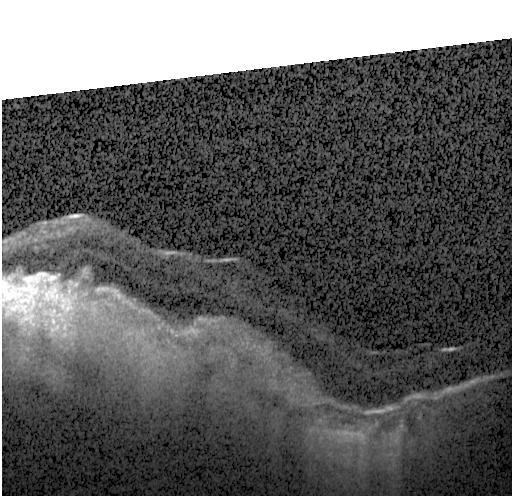 Spectral-domain OCT B-scan: CNV.